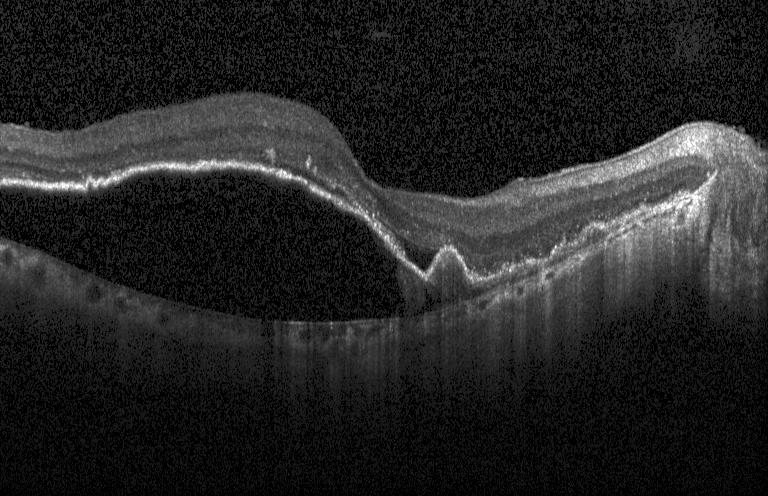 OCT finding: CNV.